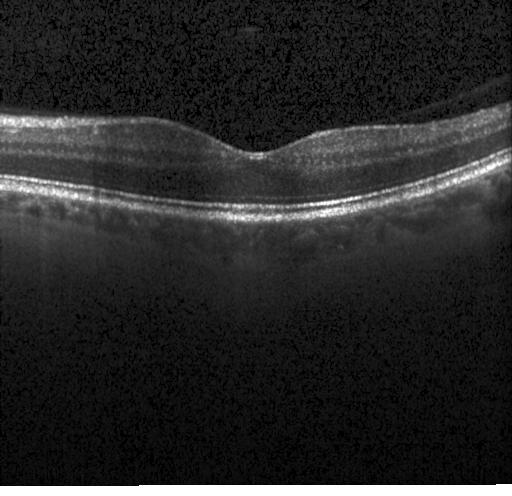

Retinal OCT cross-section. Finding: no choroidal neovascularization, no diabetic macular edema, and no drusen.